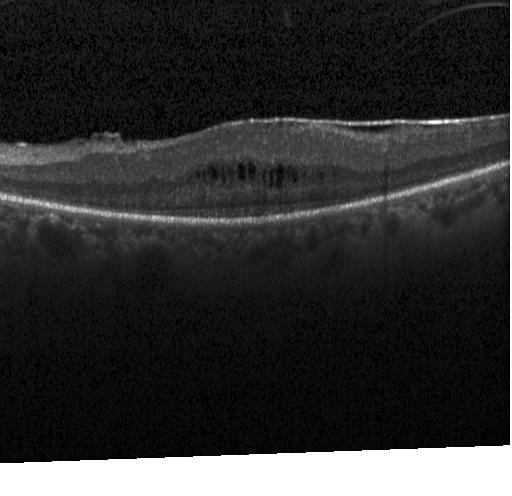

Diagnosis: diabetic macular edema (DME).